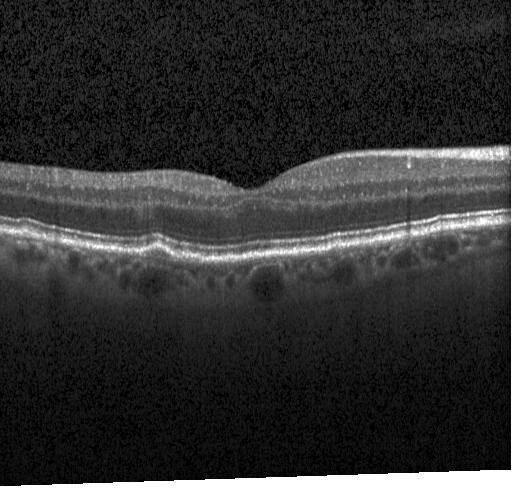 Assessment: multiple drusen.